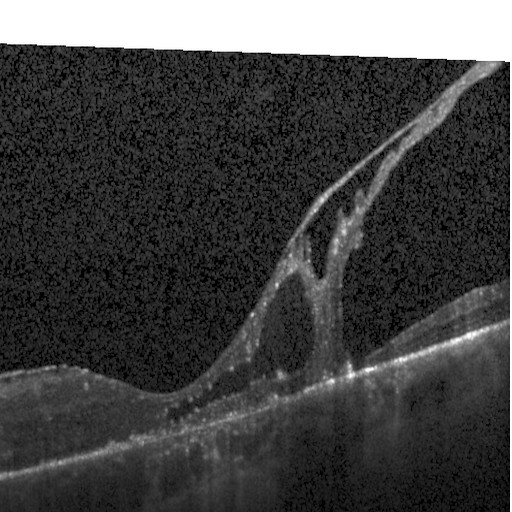
Retinal OCT B-scan · horizontal scan through the fovea · Heidelberg Spectralis.
Macular OCT: diabetic macular edema (DME).